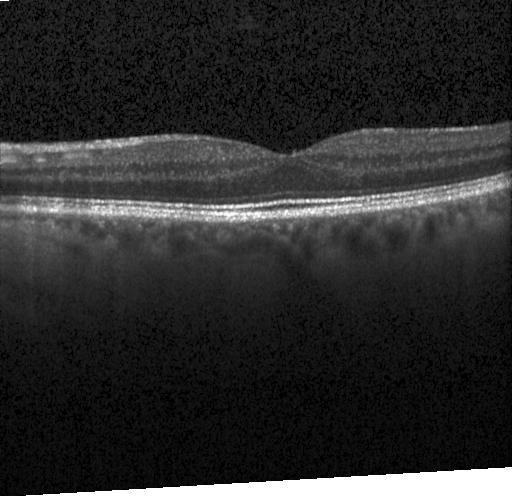
Diagnosis: no CNV, DME, or drusen.